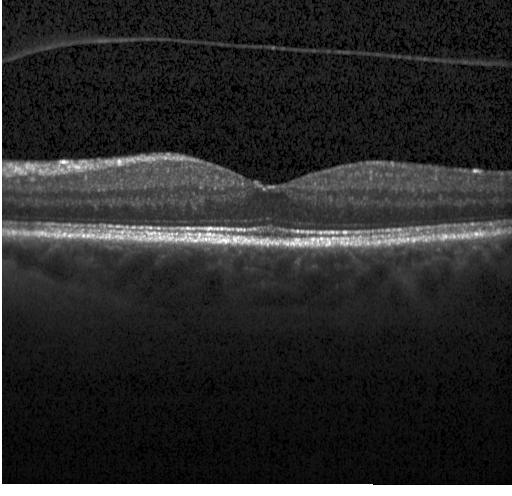 Spectral-domain OCT, OCT line scan, acquired on a Heidelberg Spectralis. Diagnosis: no evidence of choroidal neovascularization, diabetic macular edema, or drusen.